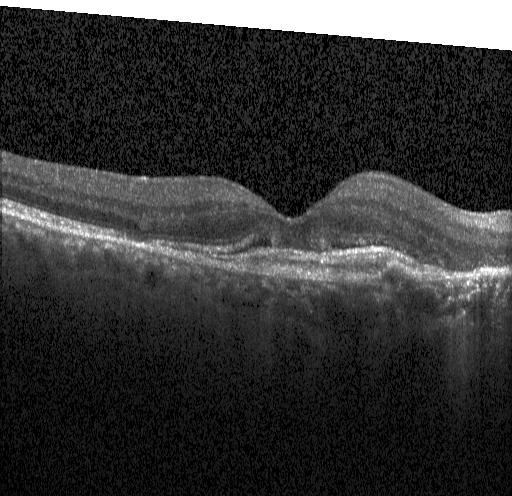 Impression: a choroidal neovascular membrane.